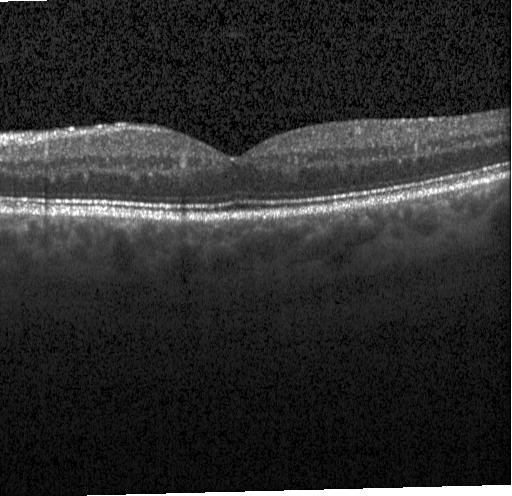
Optical coherence tomography scan.
This B-scan demonstrates no evidence of choroidal neovascularization, diabetic macular edema, or drusen.